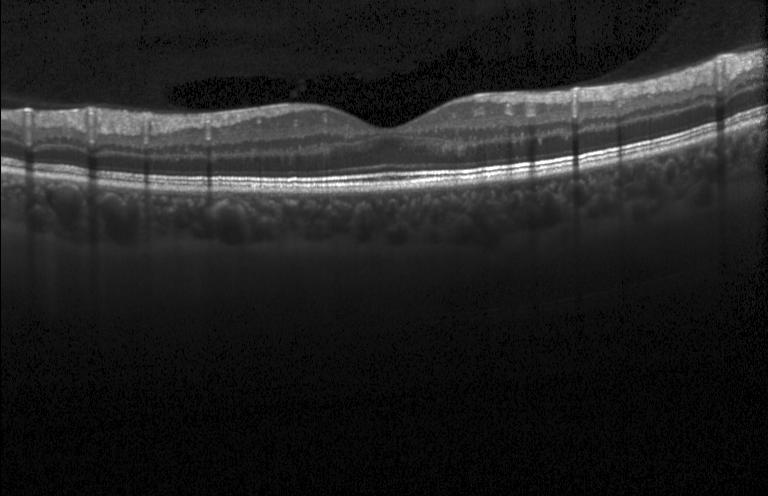 Centered on the fovea, Heidelberg Spectralis OCT system, SD-OCT, retinal OCT cross-section
This B-scan demonstrates no evidence of CNV, DME, or drusen.